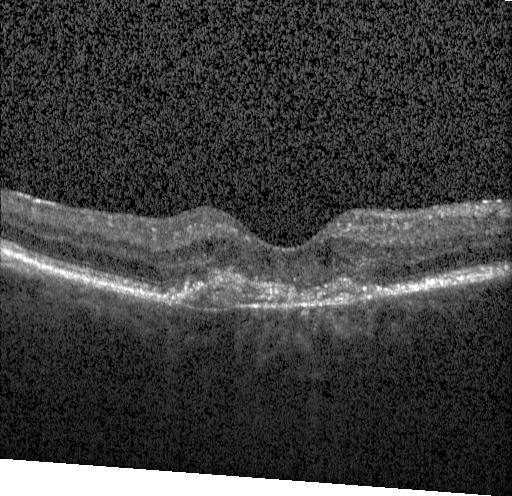

Optical coherence tomography scan.
Finding: a choroidal neovascular membrane.